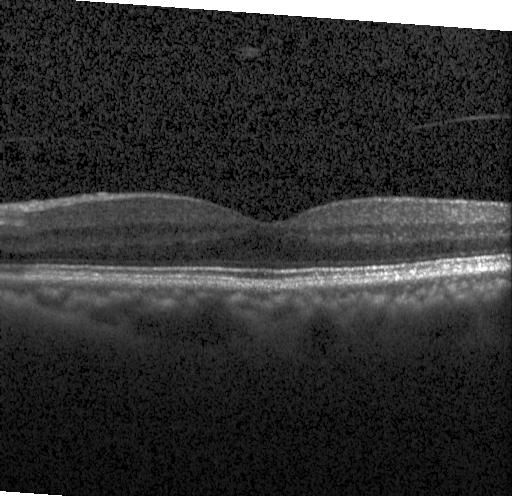
OCT line scan · instrument: Heidelberg Spectralis — OCT finding: no CNV, DME, or drusen.